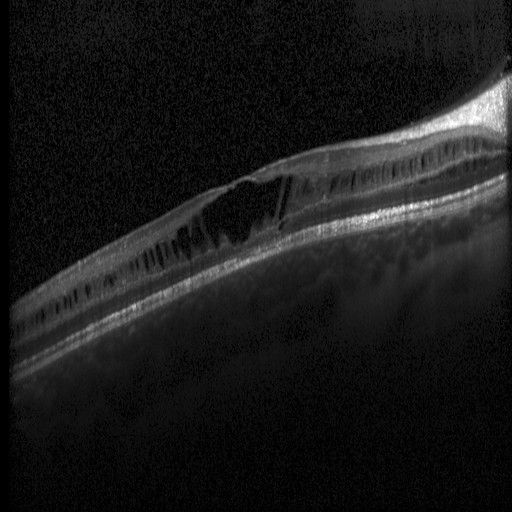
Impression: diabetic macular edema.